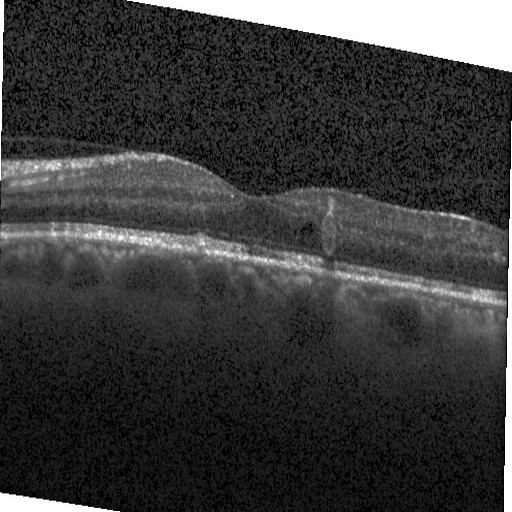

Spectral-domain optical coherence tomography, centered on the fovea, OCT B-scan.
Diabetic macular edema.